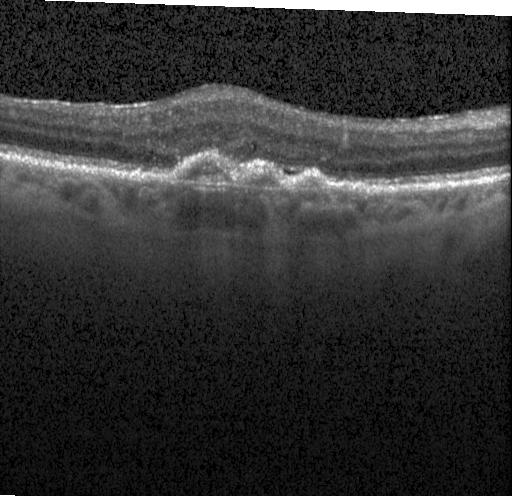

Finding: choroidal neovascularization (CNV).